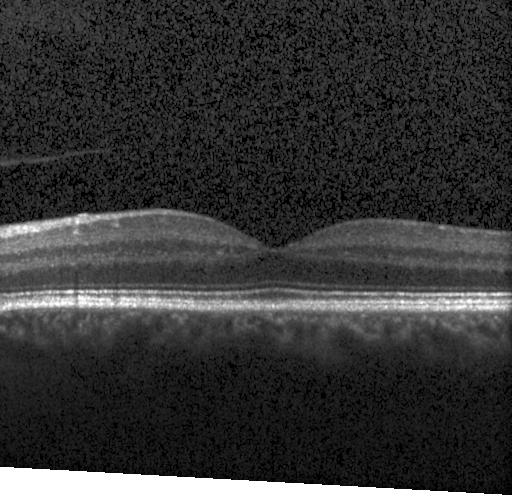 Finding: no CNV, no DME, and no drusen.